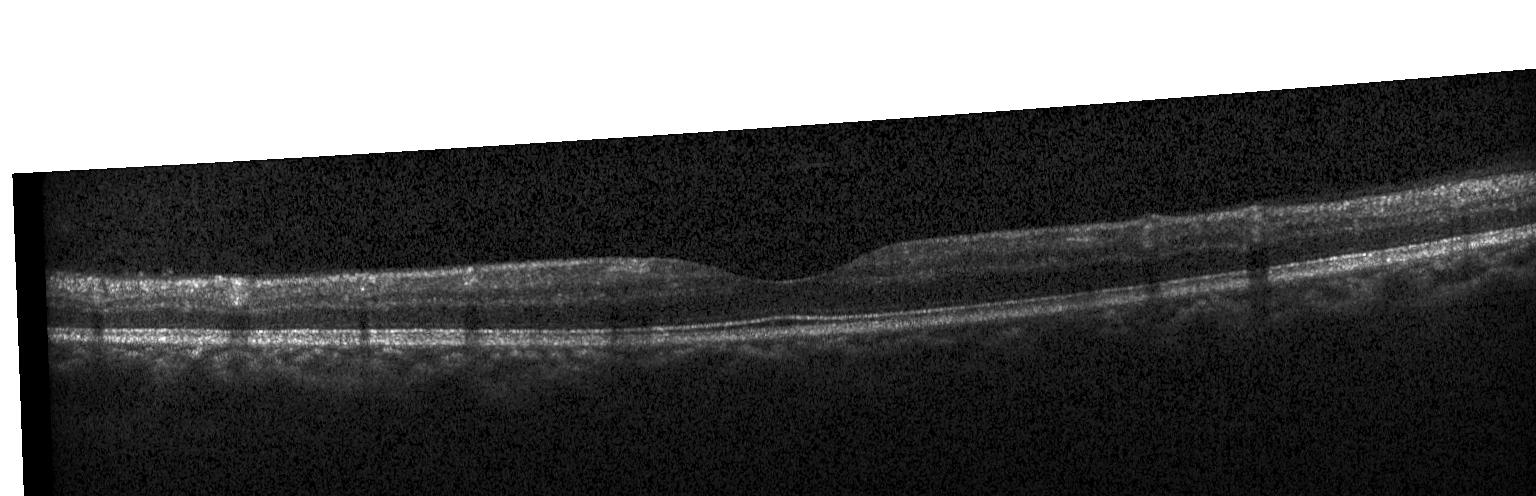 OCT B-scan
OCT finding: neither choroidal neovascularization, diabetic macular edema, nor drusen.